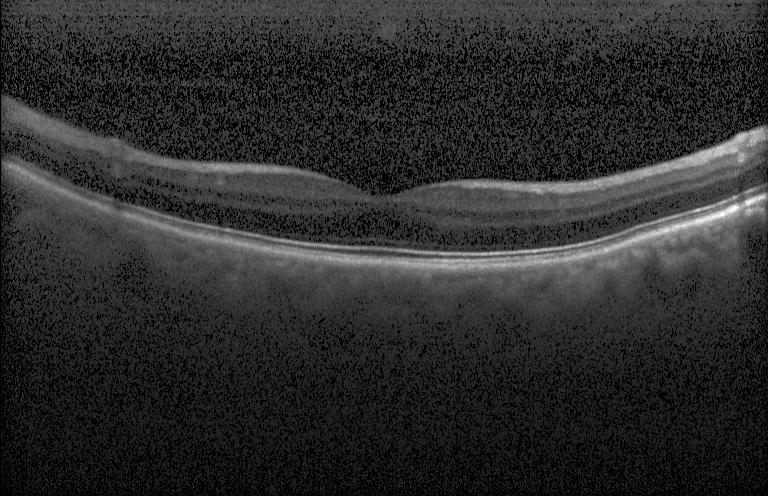
Spectral-domain optical coherence tomography · Heidelberg Spectralis · optical coherence tomography scan.
Dx: no evidence of choroidal neovascularization, diabetic macular edema, or drusen.